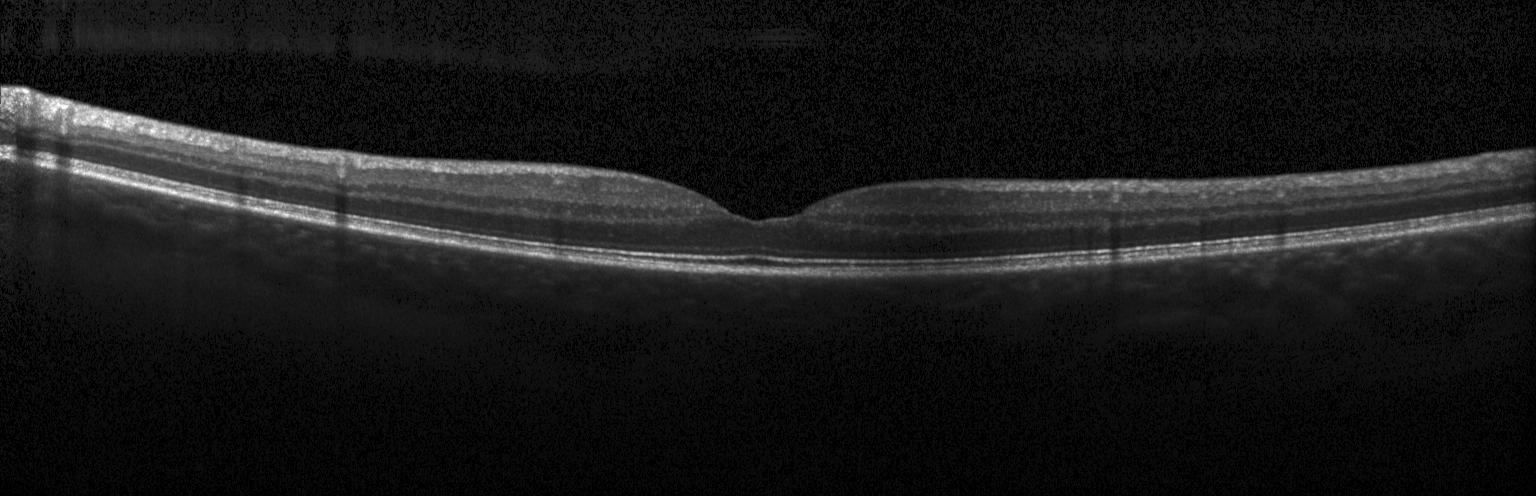

Macular OCT: no choroidal neovascularization, diabetic macular edema, or drusen.